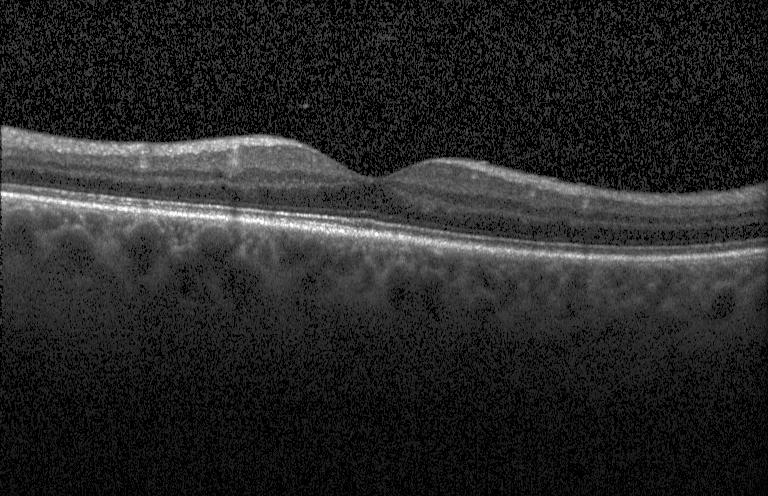
Optical coherence tomography scan — Diagnosis: no choroidal neovascularization, no diabetic macular edema, and no drusen.